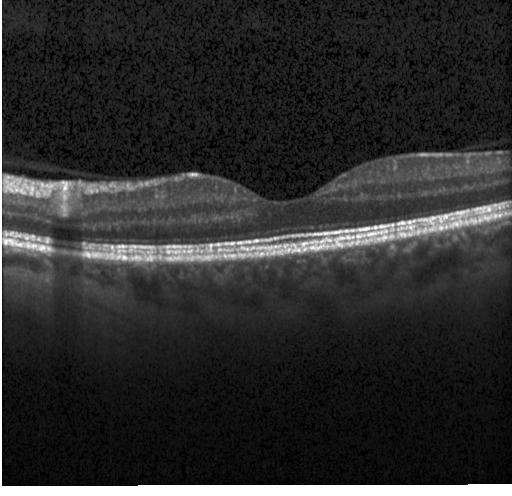 The scan shows no evidence of CNV, DME, or drusen.